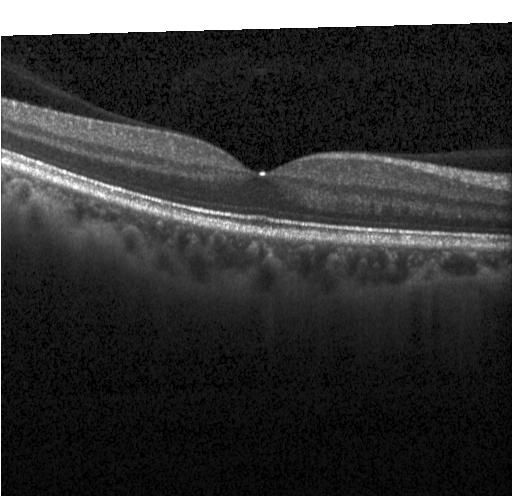
Macular scan, OCT B-scan, spectral-domain optical coherence tomography.
Assessment: neither CNV, DME, nor drusen.